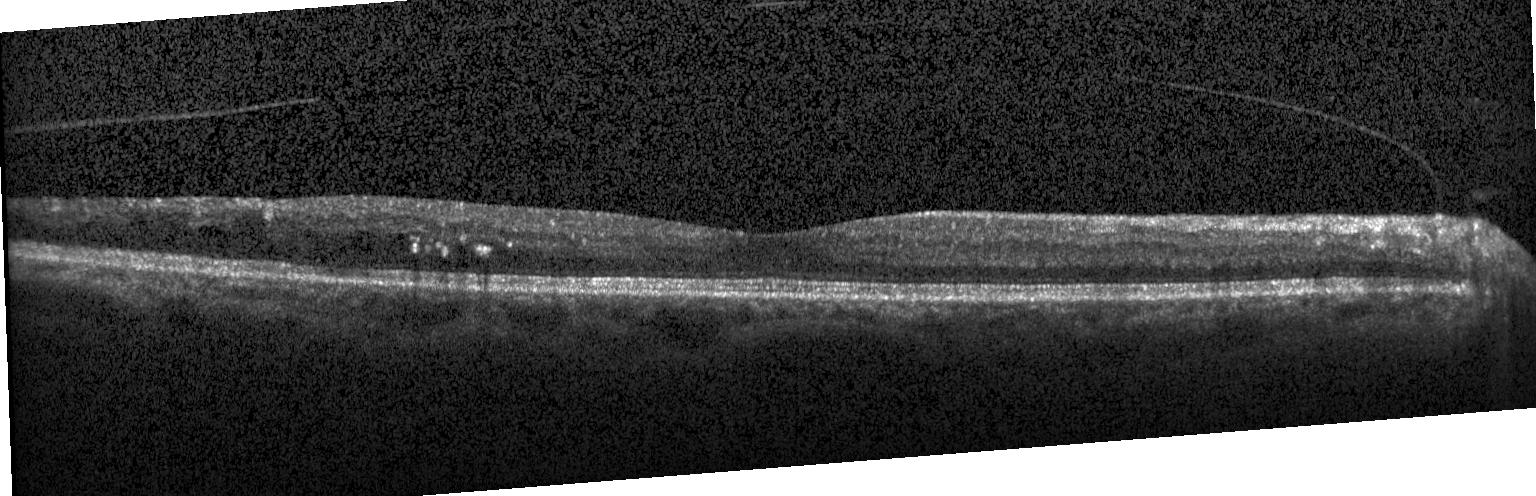
Retinal OCT cross-section.
Finding: diabetic macular edema.